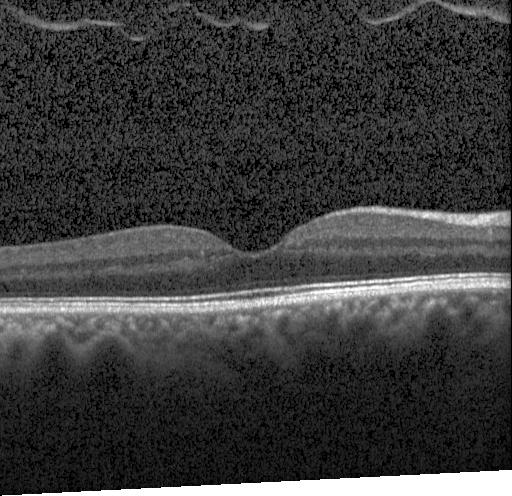 Spectral-domain OCT B-scan: no CNV, no DME, and no drusen.